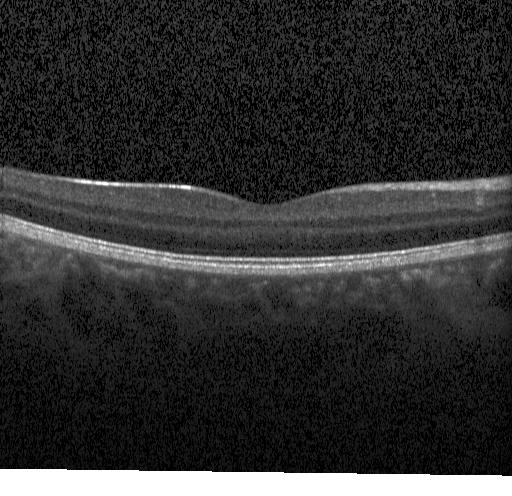

Optical coherence tomography scan. Spectral-domain OCT. Finding: no evidence of choroidal neovascularization, diabetic macular edema, or drusen.